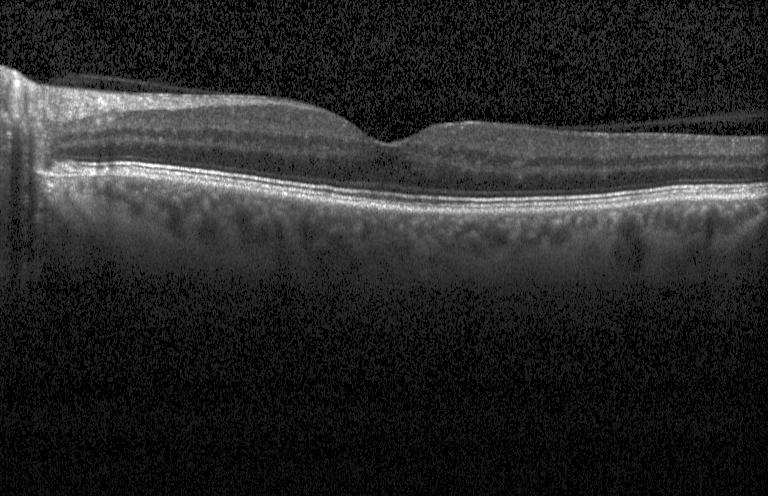 No choroidal neovascularization, no diabetic macular edema, and no drusen.